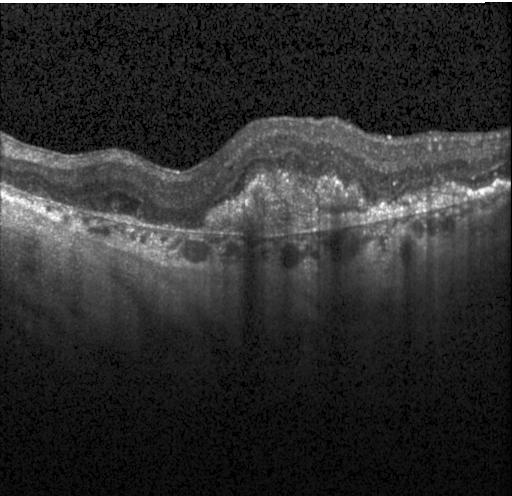

OCT B-scan.
Impression: a choroidal neovascular membrane.